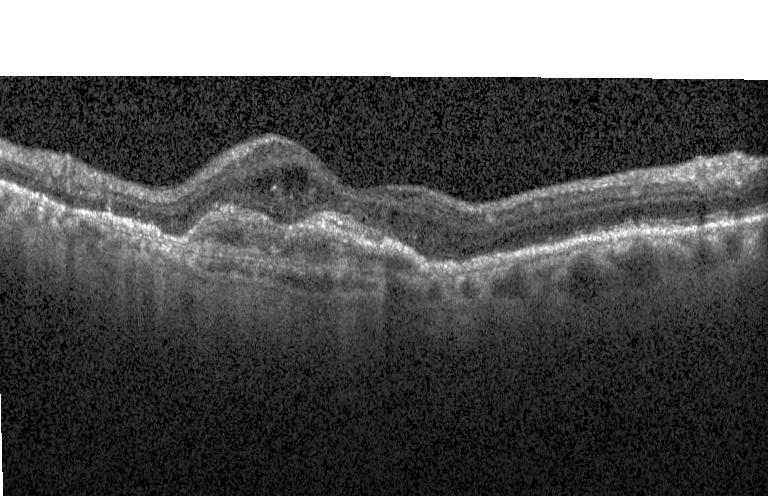

OCT B-scan. Choroidal neovascularization.